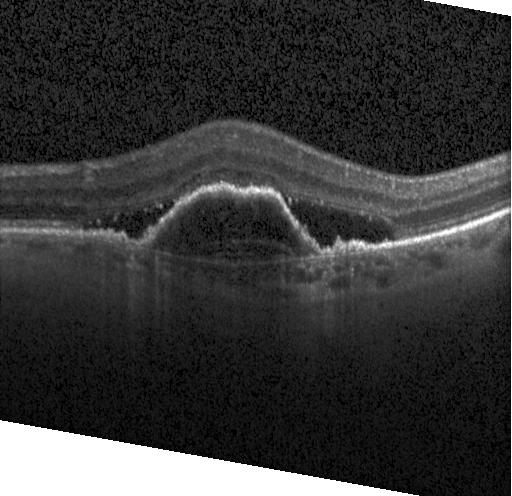
Retinal OCT B-scan
Finding: a choroidal neovascular membrane.